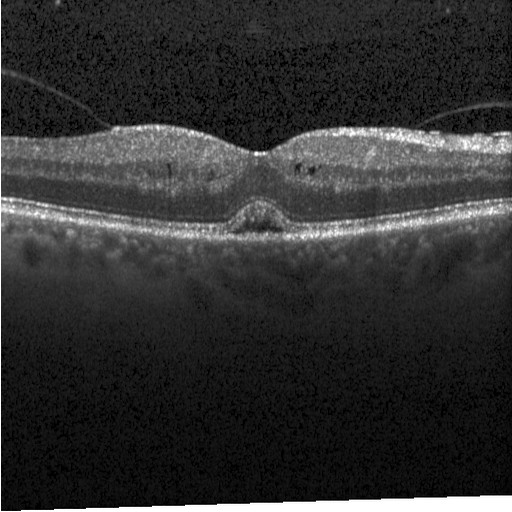
Retinal OCT B-scan — Impression: diabetic macular edema (DME).